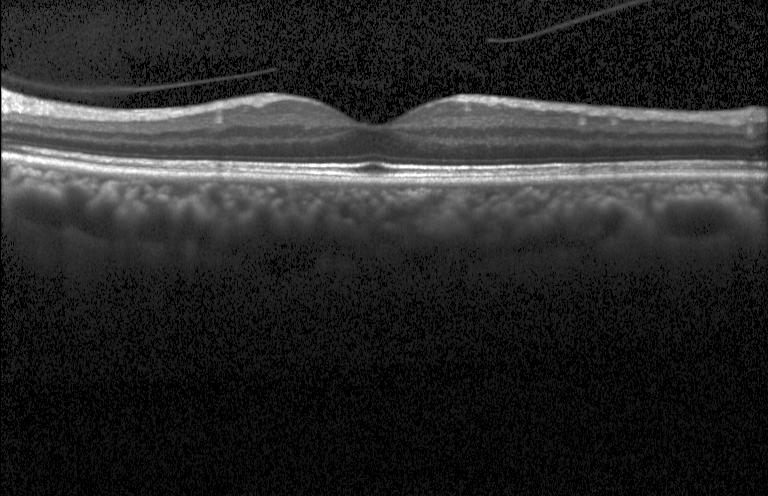
Optical coherence tomography scan. Heidelberg Spectralis OCT system — This B-scan demonstrates neither CNV, DME, nor drusen.